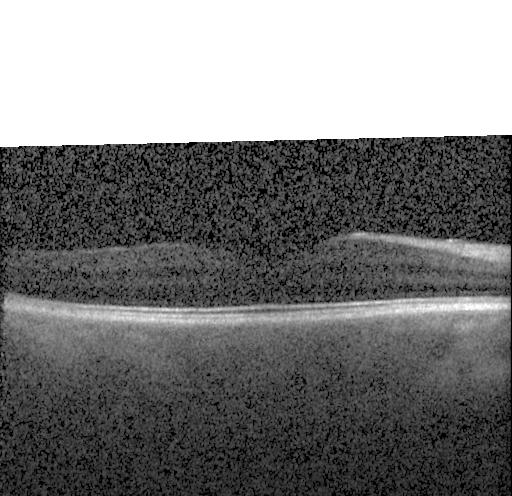 Retinal OCT cross-section showing no CNV, DME, or drusen.